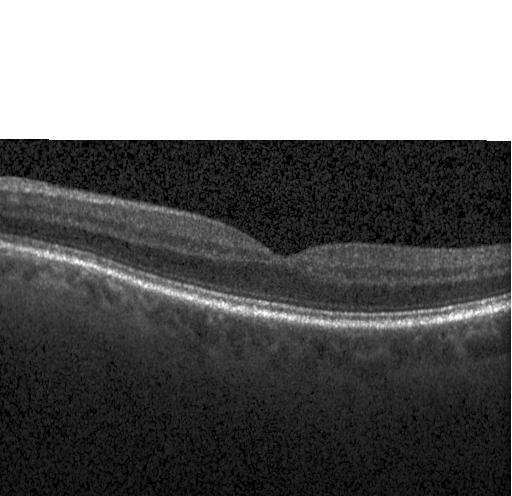 OCT B-scan showing neither CNV, DME, nor drusen.